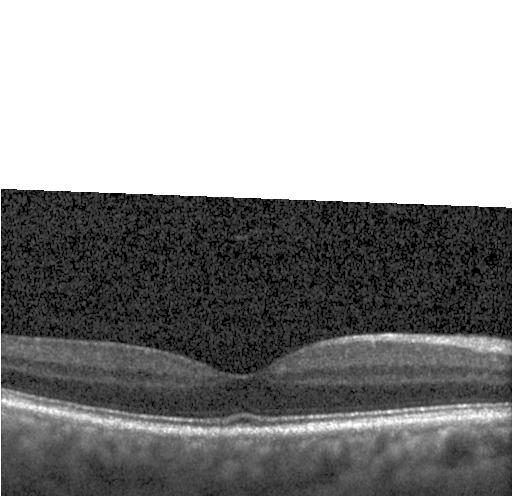

Diagnosis: no CNV, no DME, and no drusen.